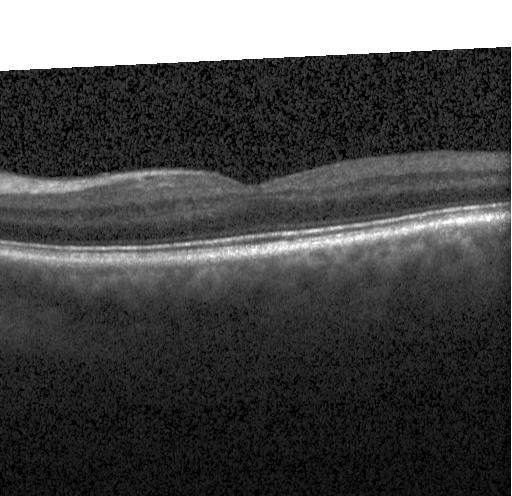 Heidelberg Spectralis OCT system, optical coherence tomography scan, spectral-domain OCT, fovea-centered. Macular OCT: no evidence of CNV, DME, or drusen.